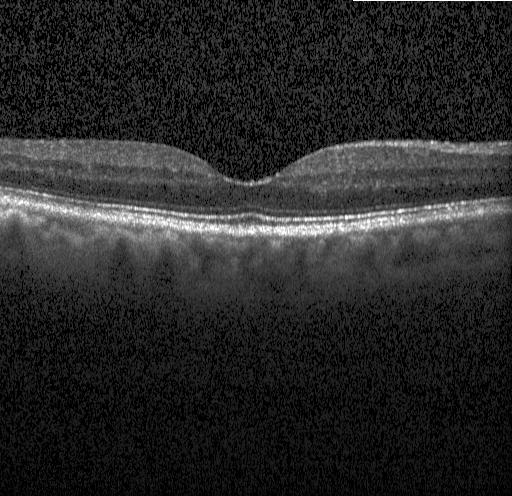
Centered on the fovea. Heidelberg Spectralis. OCT line scan
Diagnosis: no evidence of choroidal neovascularization, diabetic macular edema, or drusen.